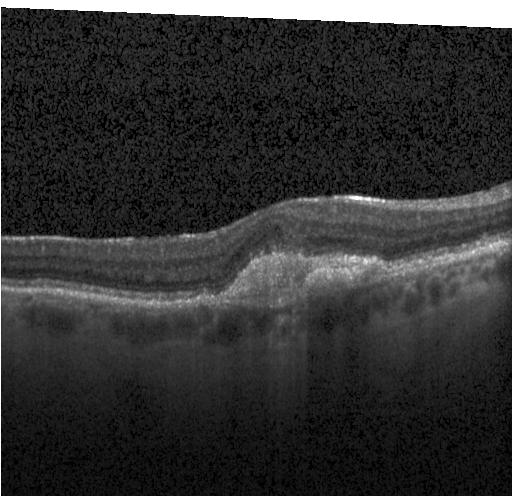
OCT finding: a choroidal neovascular membrane.